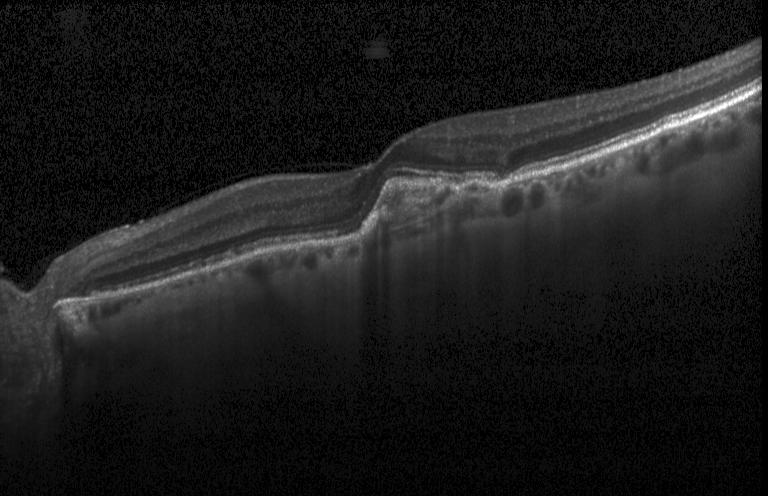

Optical coherence tomography B-scan · through the macula · SD-OCT · instrument: Heidelberg Spectralis. Assessment: choroidal neovascularization.